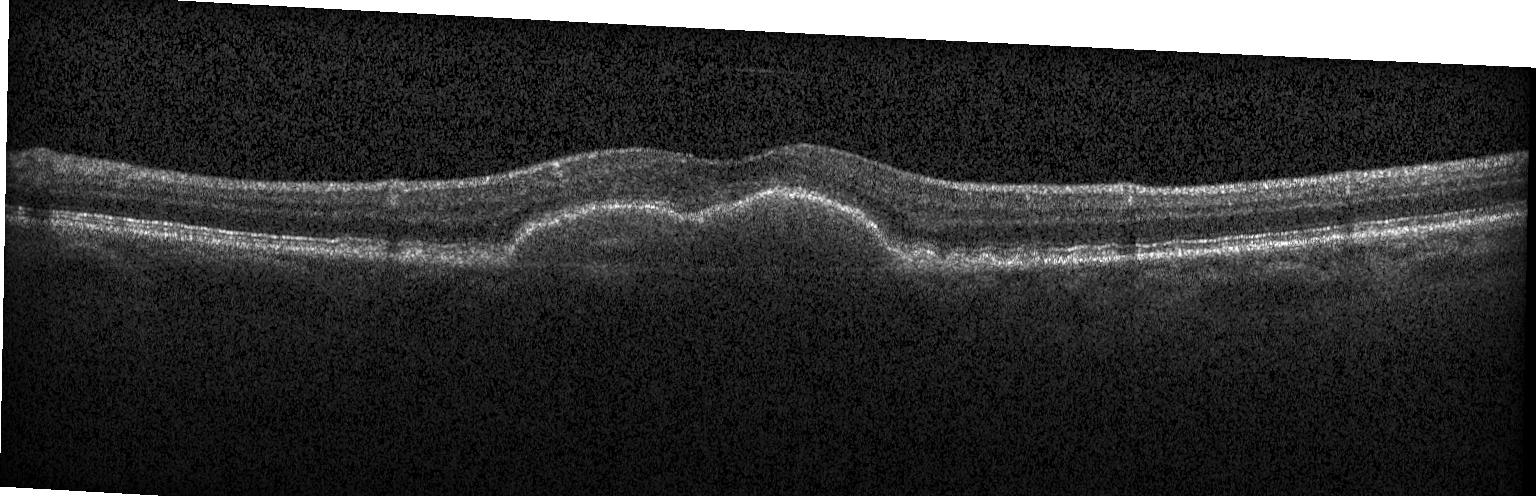
Spectral-domain OCT B-scan: CNV.